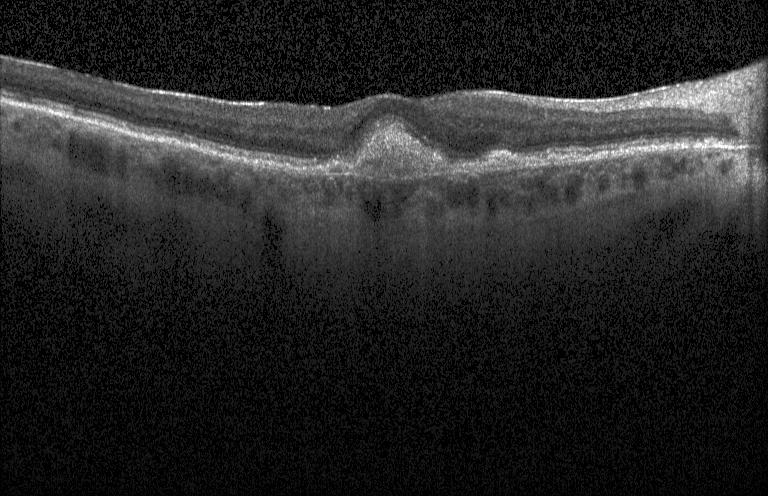

Acquired on a Heidelberg Spectralis · retinal OCT B-scan · centered on the fovea · SD-OCT. Diagnosis: a choroidal neovascular membrane.